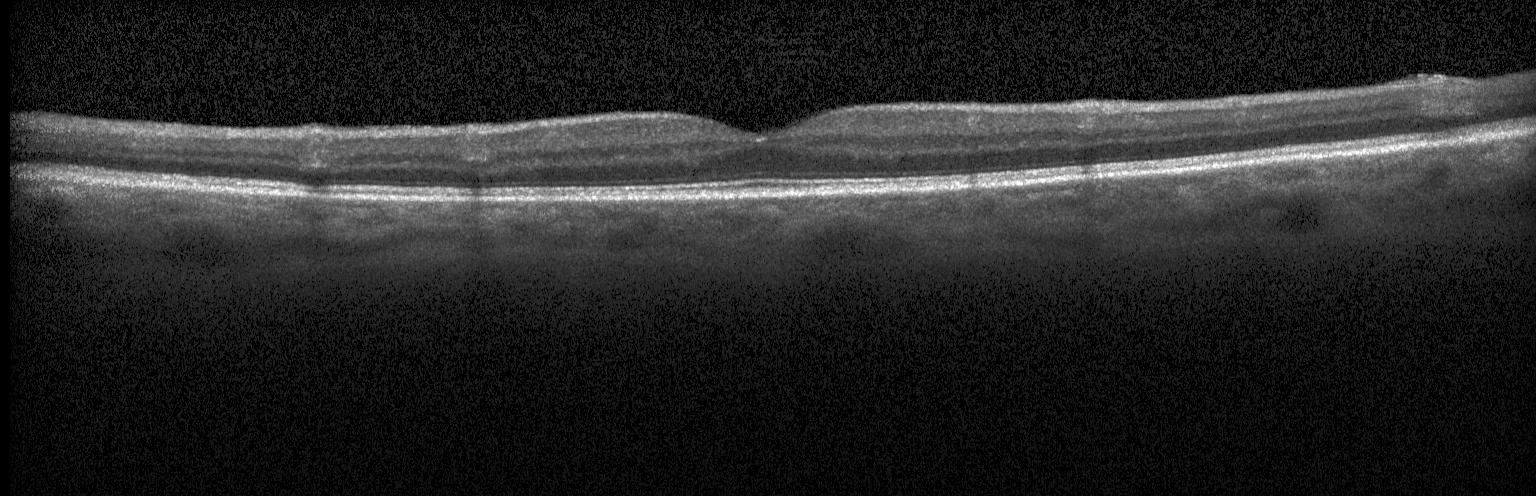
Optical coherence tomography B-scan.
Macular OCT: no evidence of CNV, DME, or drusen.